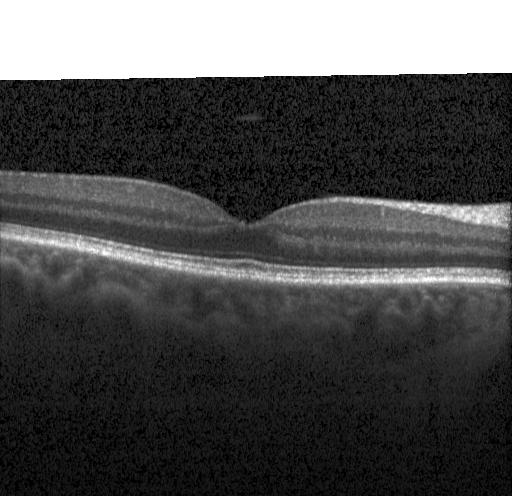 OCT B-scan. Spectral-domain optical coherence tomography. Through the macula. Instrument: Heidelberg Spectralis. Diagnosis: neither CNV, DME, nor drusen.